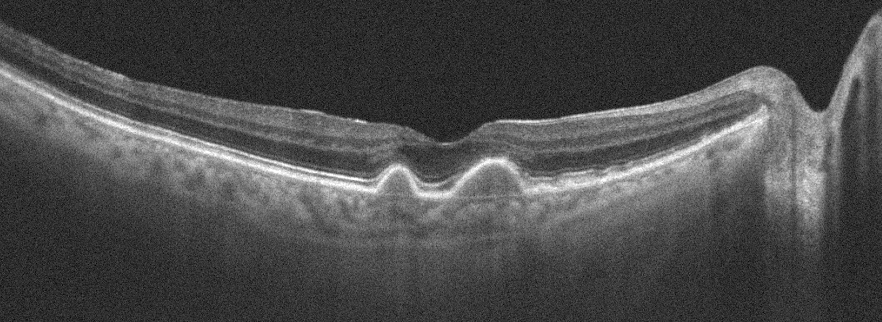 OCT line scan. OD
Impression: AMD.